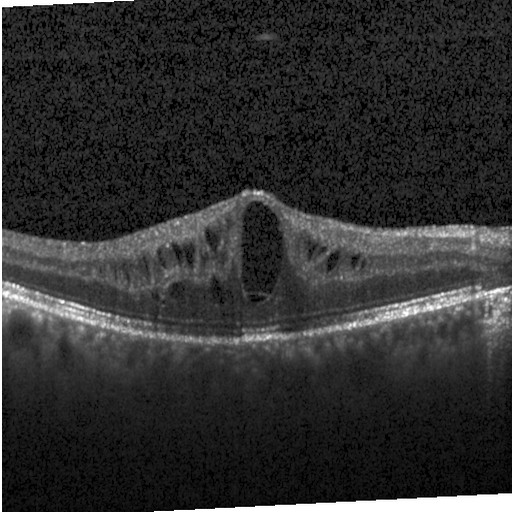 Macular scan, optical coherence tomography B-scan, instrument: Heidelberg Spectralis. Macular OCT: diabetic macular edema (DME).